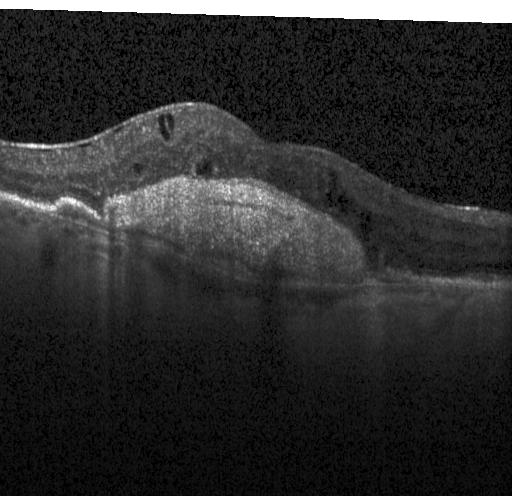

Dx: a choroidal neovascular membrane.